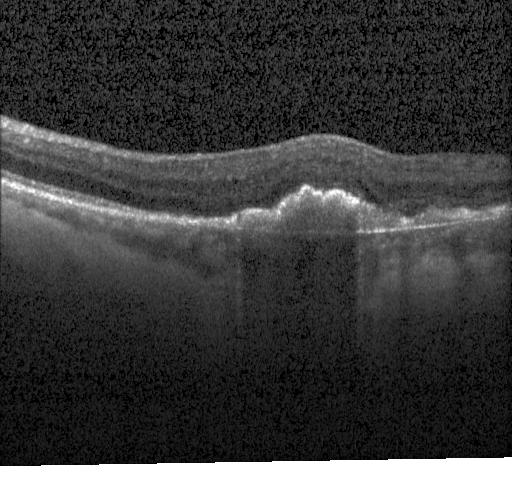
Spectral-domain optical coherence tomography. Heidelberg Spectralis. Horizontal scan through the fovea. Retinal OCT B-scan
This B-scan demonstrates a choroidal neovascular membrane.